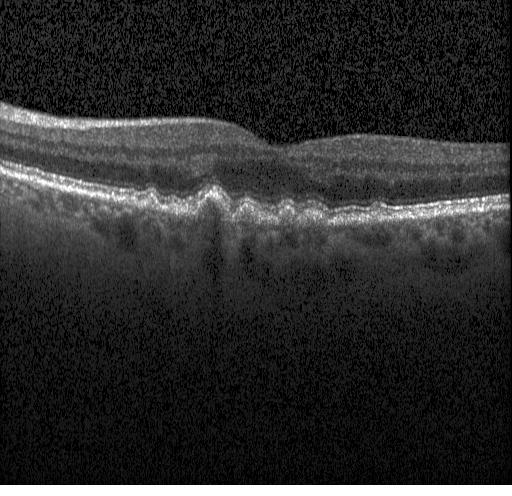
Retinal OCT cross-section — Diagnosis: multiple drusen.